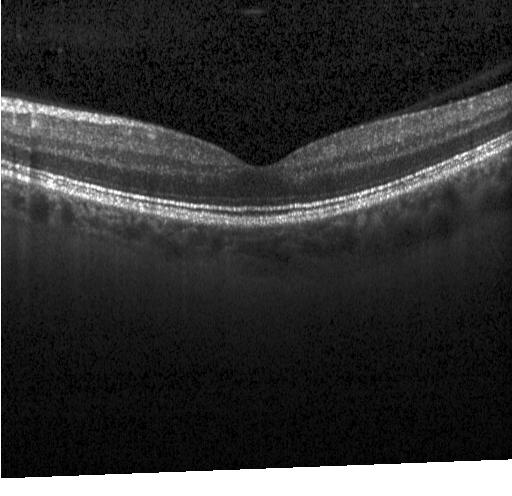 Centered on the fovea · optical coherence tomography scan. Assessment: no CNV, DME, or drusen.